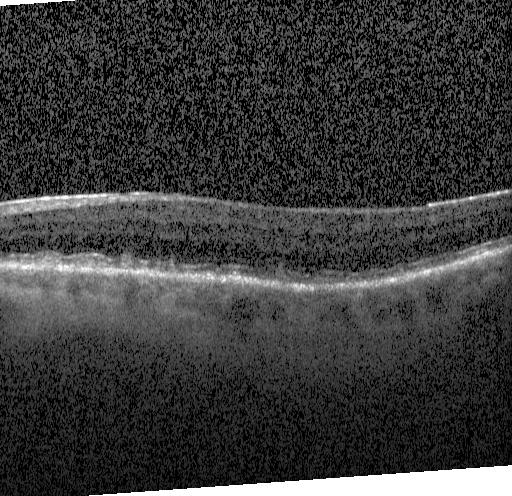
OCT B-scan showing sub-RPE drusenoid deposits.